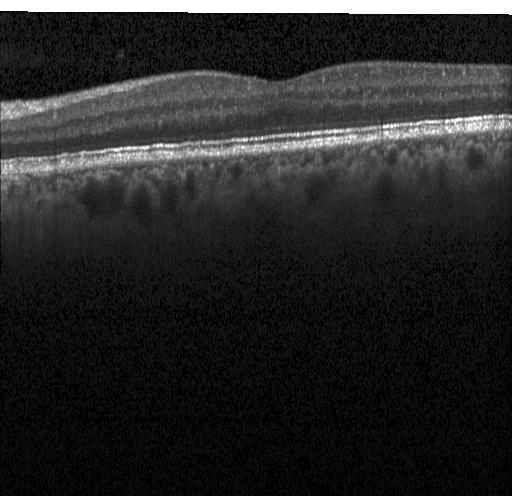 Optical coherence tomography scan. Heidelberg Spectralis OCT system. Through the macula.
Assessment: no choroidal neovascularization, diabetic macular edema, or drusen.